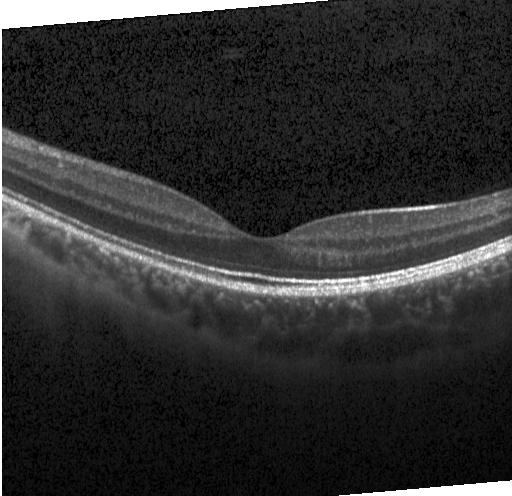
Retinal OCT cross-section; through the macula. Impression: neither choroidal neovascularization, diabetic macular edema, nor drusen.